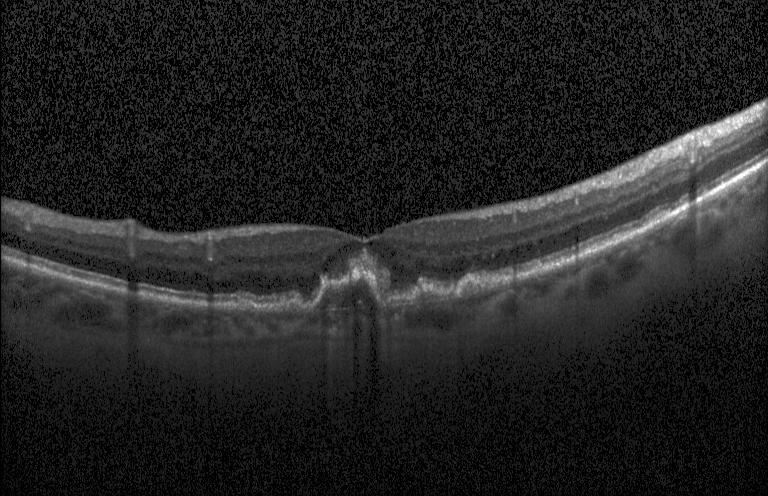

Macular OCT demonstrating a choroidal neovascular membrane.